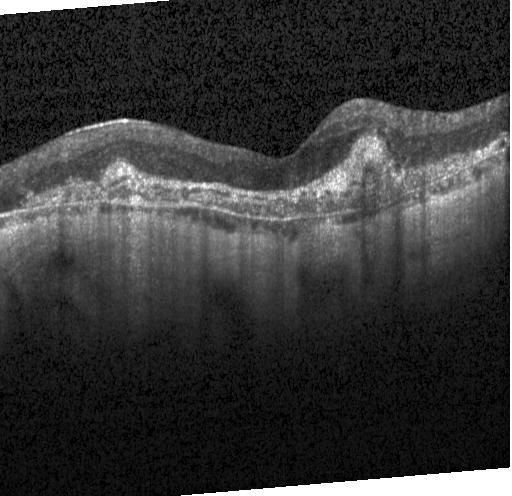 Diagnosis: a choroidal neovascular membrane.